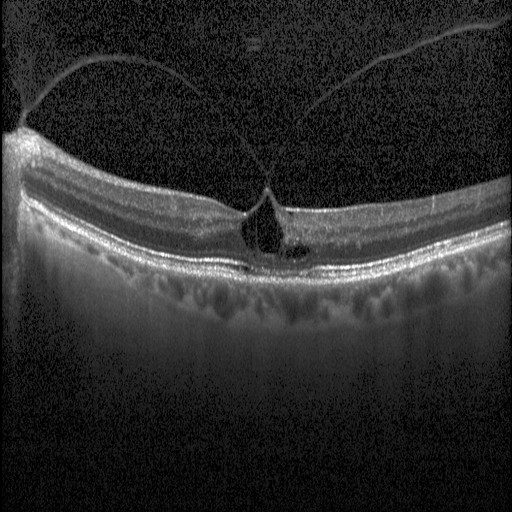

Retinal OCT B-scan.
This B-scan demonstrates DME.